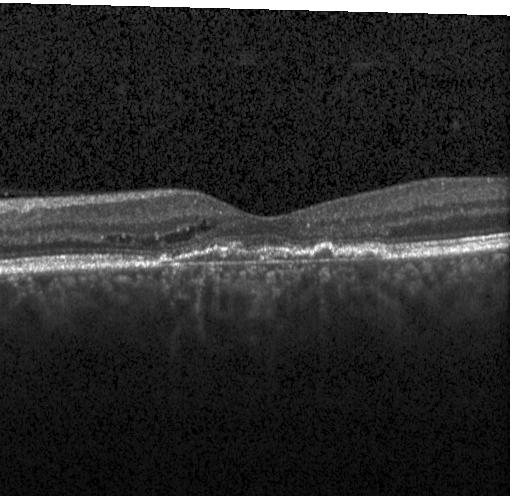 Assessment: choroidal neovascularization (CNV).